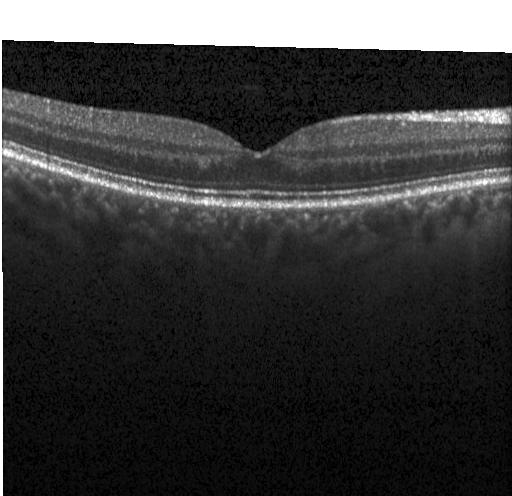
Spectral-domain OCT B-scan: no CNV, DME, or drusen.